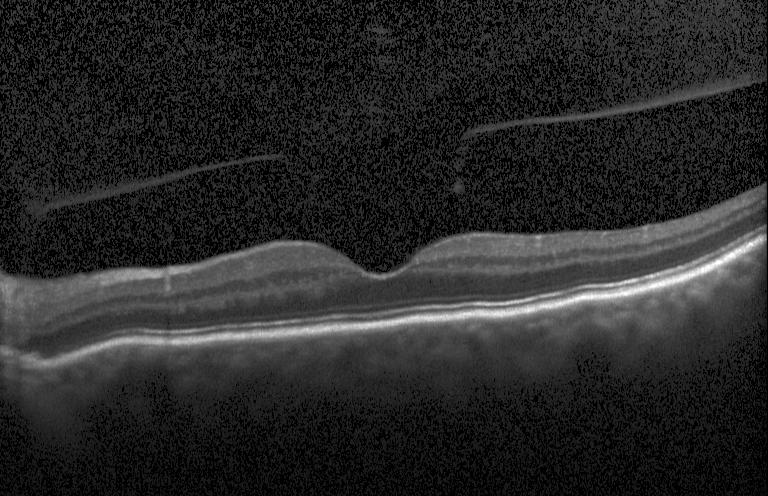
OCT line scan, spectral-domain optical coherence tomography.
Impression: no choroidal neovascularization, no diabetic macular edema, and no drusen.